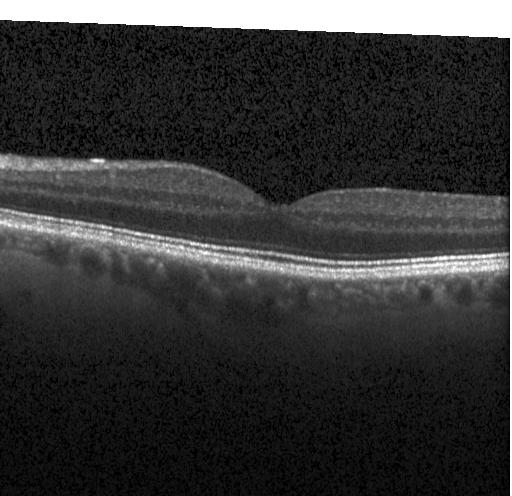 Optical coherence tomography scan. The scan shows neither choroidal neovascularization, diabetic macular edema, nor drusen.